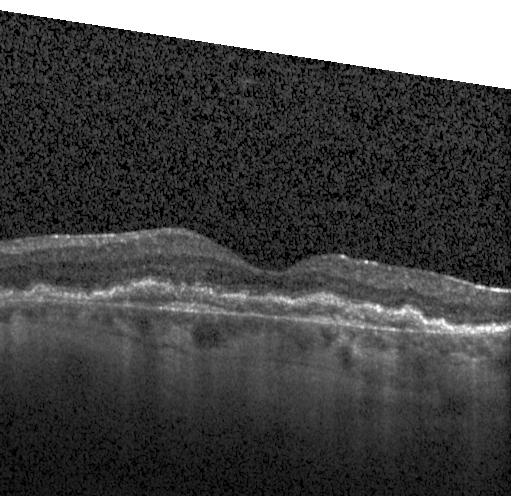
Macular OCT: a choroidal neovascular membrane.